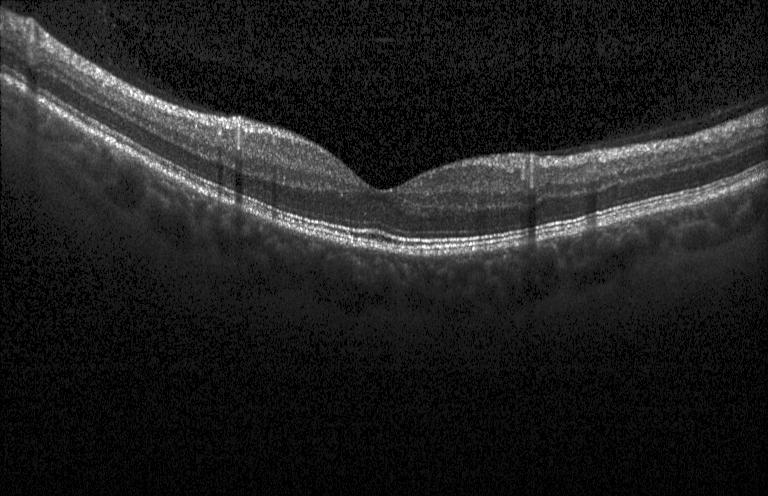
Heidelberg Spectralis. Centered on the fovea. Spectral-domain OCT. Optical coherence tomography scan. No evidence of choroidal neovascularization, diabetic macular edema, or drusen.